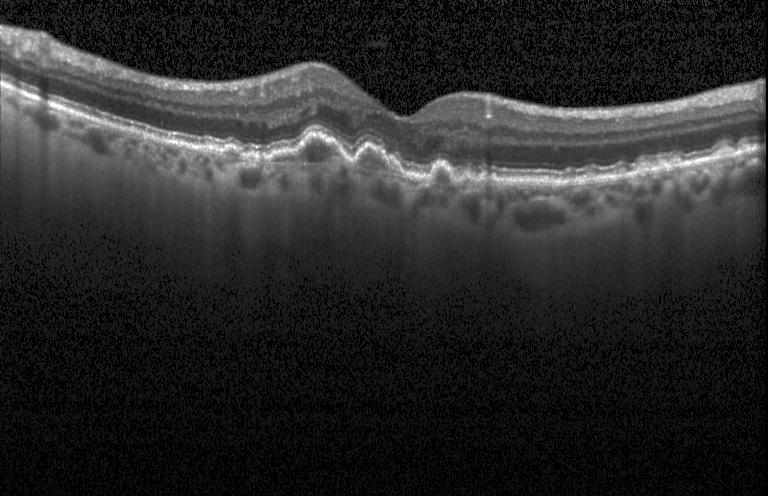

Retinal OCT cross-section, centered on the fovea.
A choroidal neovascular membrane.